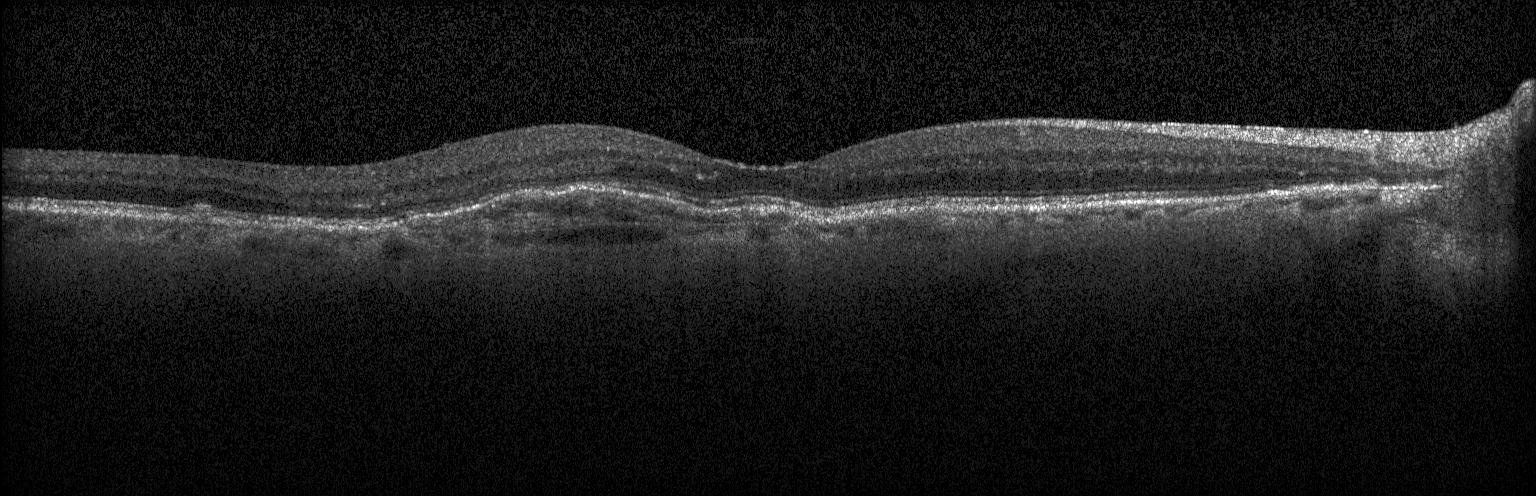

Finding: a choroidal neovascular membrane.